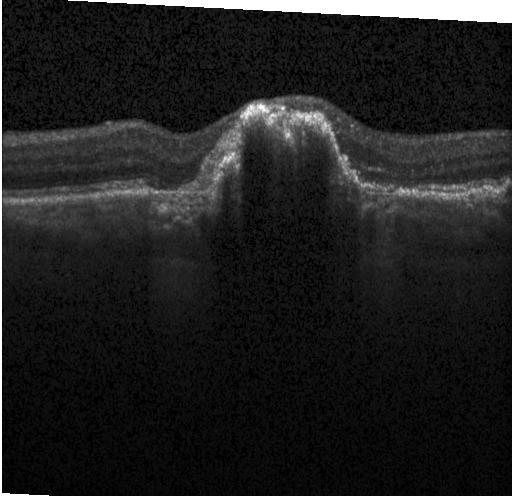

Acquired on a Heidelberg Spectralis · through the macula · optical coherence tomography scan — This B-scan demonstrates a choroidal neovascular membrane.